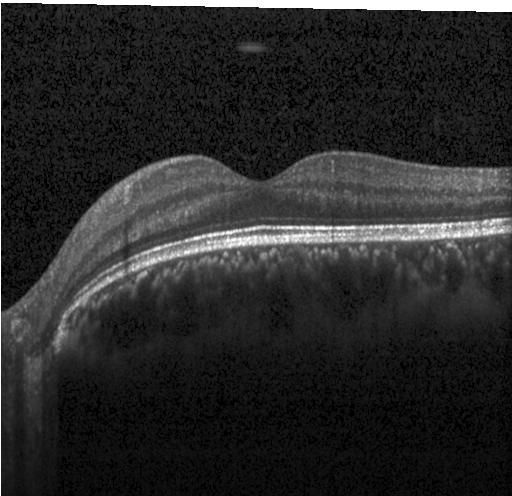 Impression: no choroidal neovascularization, no diabetic macular edema, and no drusen.